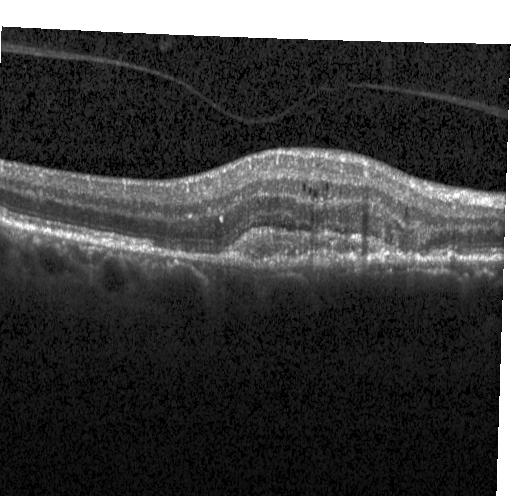 Assessment: a choroidal neovascular membrane.